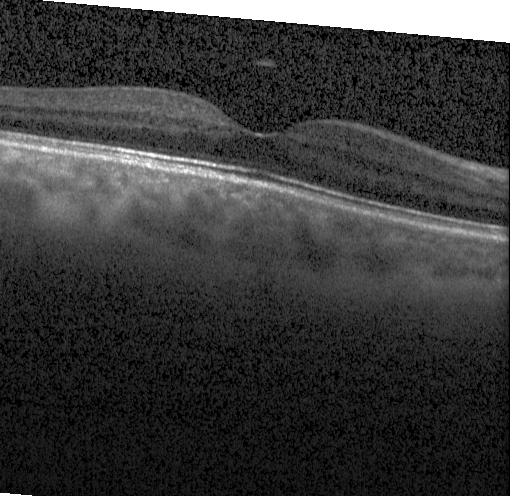
Assessment: no choroidal neovascularization, diabetic macular edema, or drusen.